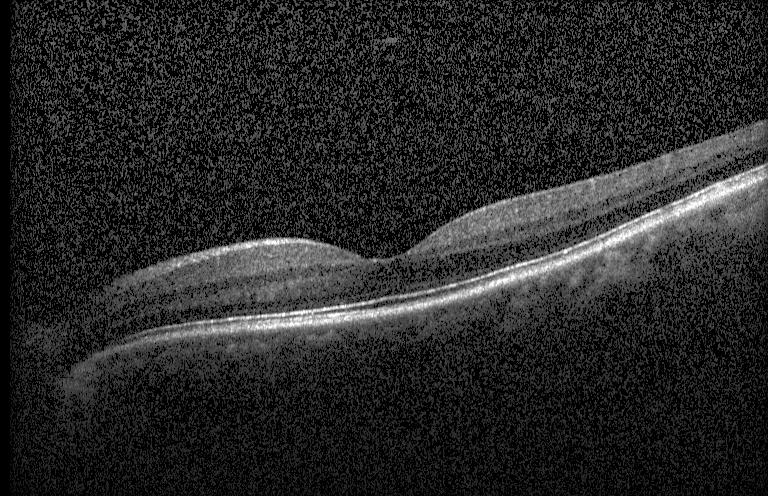
No choroidal neovascularization, diabetic macular edema, or drusen.